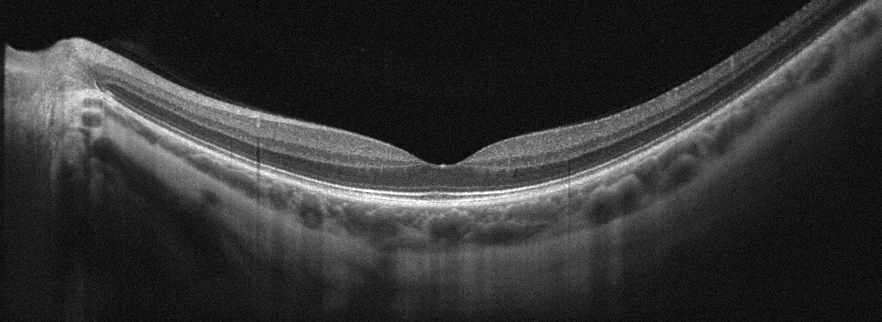
Left eye; retinal OCT B-scan; fovea-centered — Finding: absence of AMD, DME, ERM, RAO, RVO, and vitreomacular interface disease.